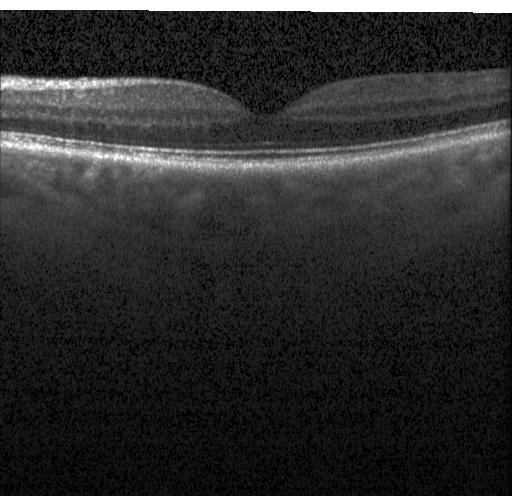 Fovea-centered, instrument: Heidelberg Spectralis, OCT line scan.
OCT finding: no choroidal neovascularization, no diabetic macular edema, and no drusen.